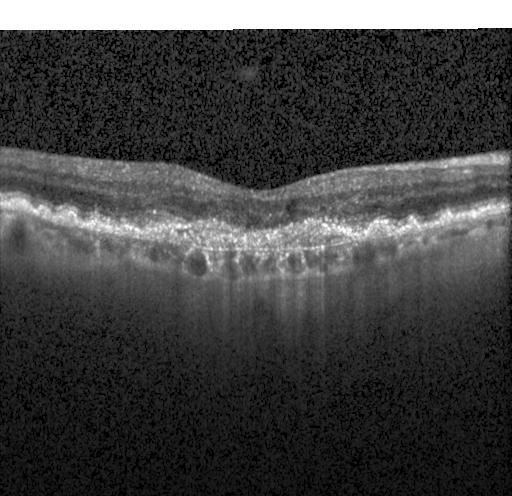

SD-OCT. OCT line scan. Centered on the fovea. Heidelberg Spectralis
Impression: choroidal neovascularization.